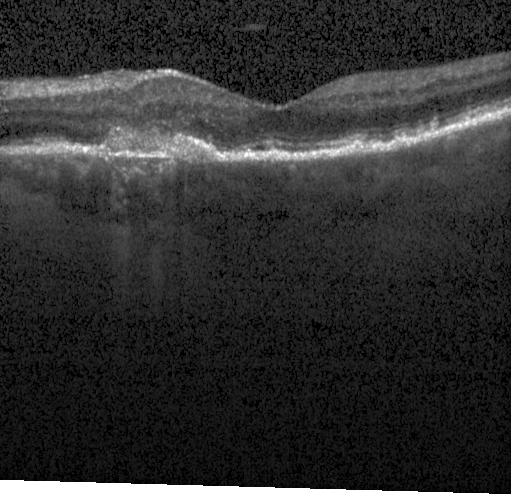
Diagnosis: a choroidal neovascular membrane.